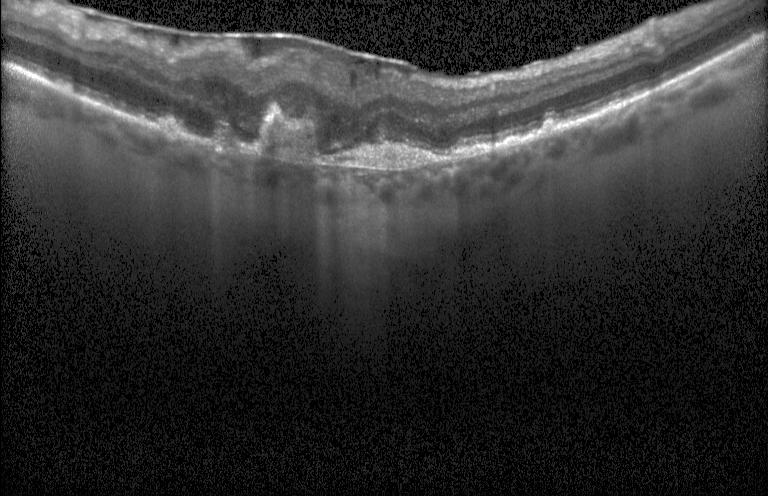
This B-scan demonstrates choroidal neovascularization (CNV).